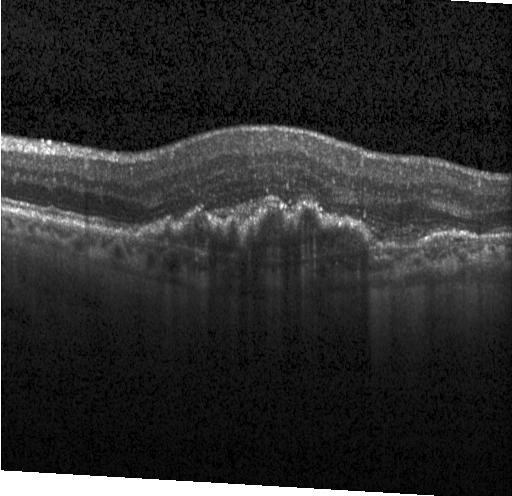 SD-OCT; OCT B-scan
Diagnosis: a choroidal neovascular membrane.